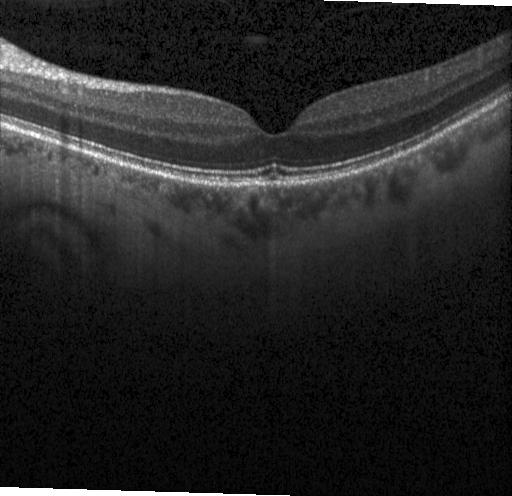
Acquired on a Heidelberg Spectralis. Spectral-domain optical coherence tomography. Optical coherence tomography B-scan.
Diagnosis: neither CNV, DME, nor drusen.